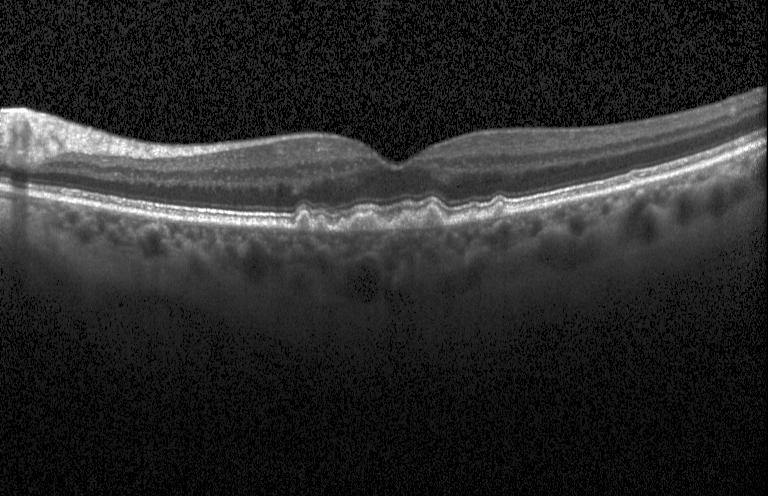 Diagnosis: sub-RPE drusenoid deposits.